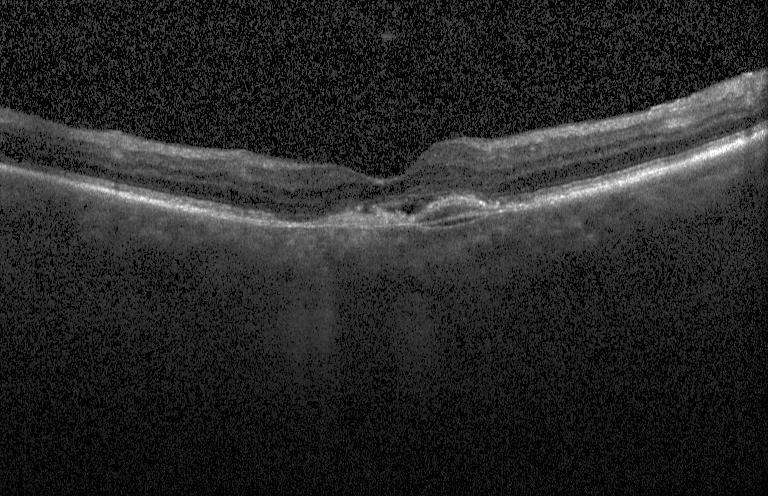

OCT finding: choroidal neovascularization (CNV).